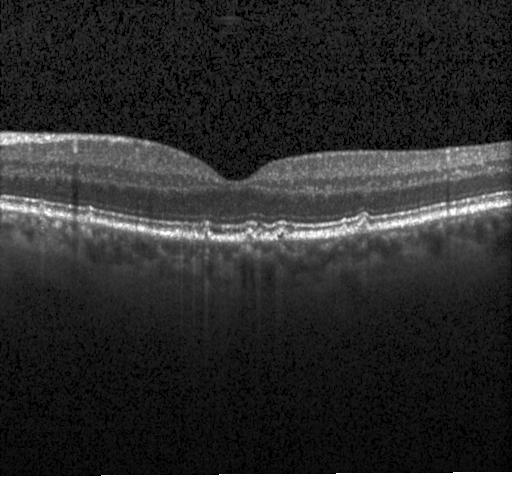

Finding: multiple drusen.